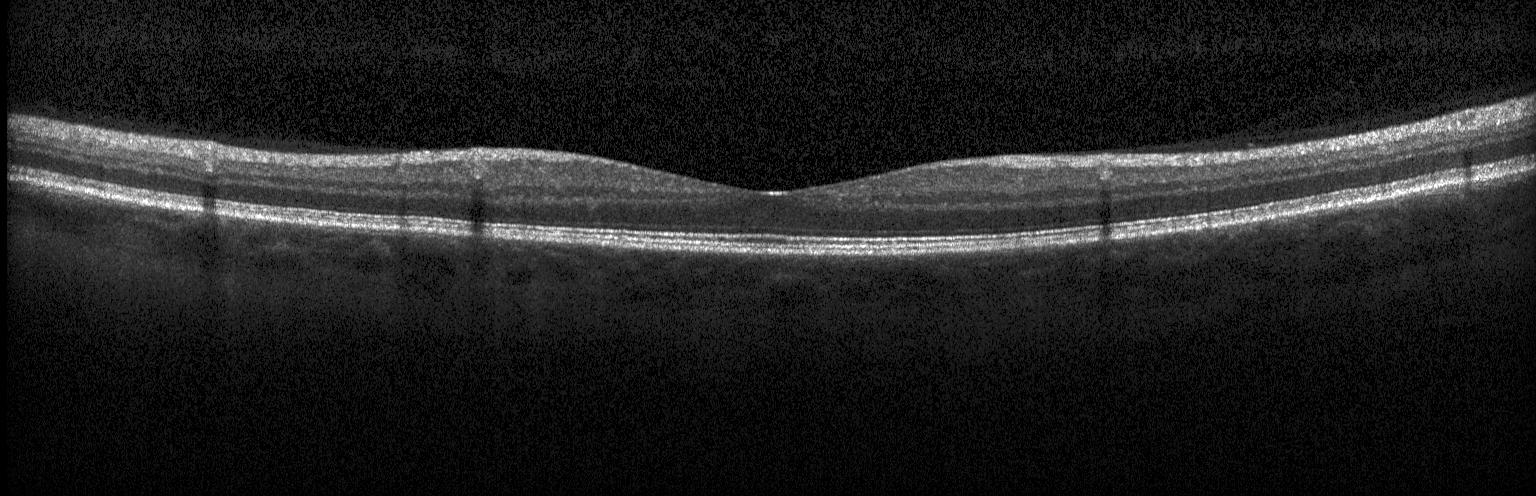

OCT B-scan, centered on the fovea, spectral-domain optical coherence tomography, acquired on a Heidelberg Spectralis — OCT finding: neither CNV, DME, nor drusen.